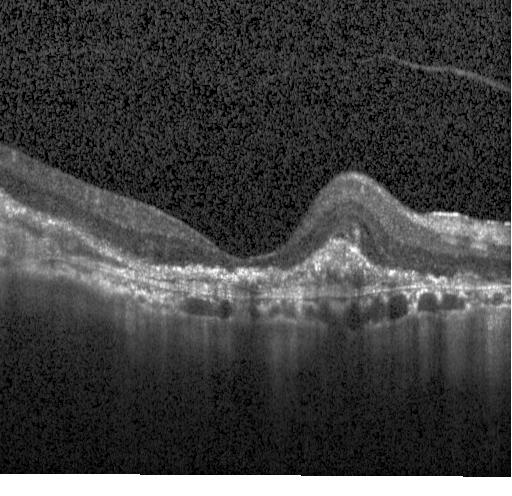
Retinal OCT cross-section showing choroidal neovascularization (CNV).